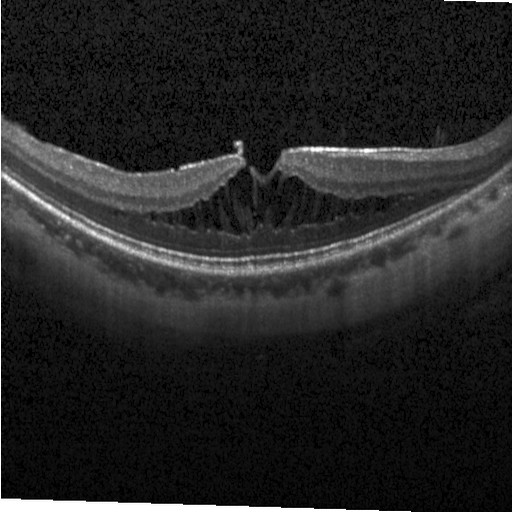

OCT scan showing diabetic macular edema.